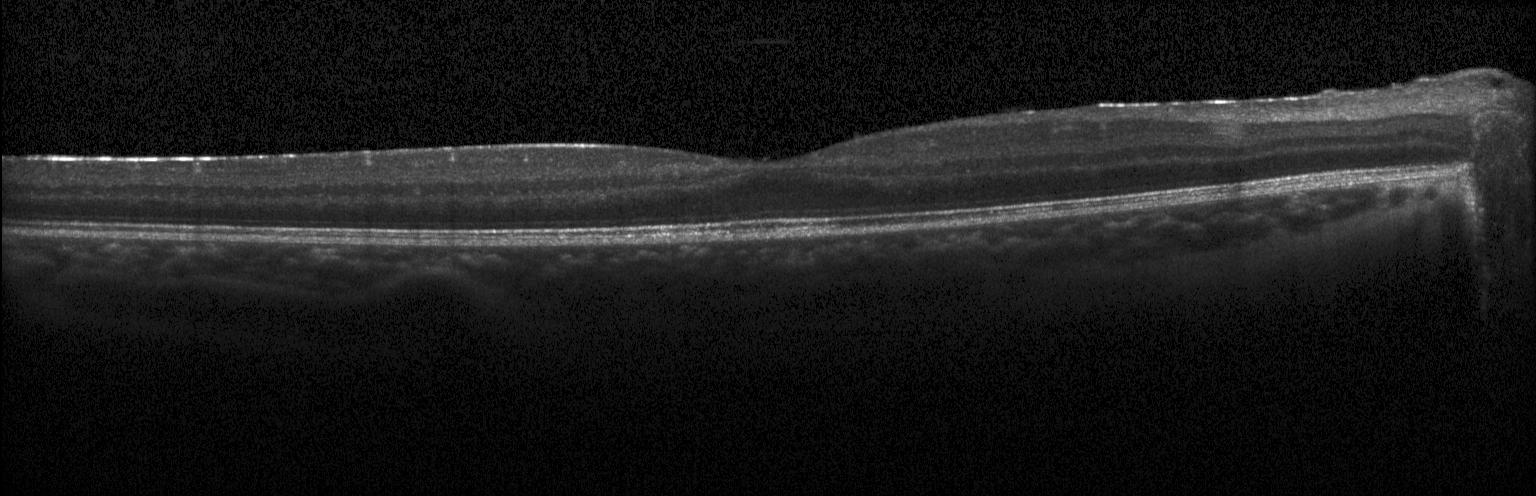 SD-OCT, through the macula, retinal OCT cross-section, Heidelberg Spectralis — OCT finding: no CNV, no DME, and no drusen.